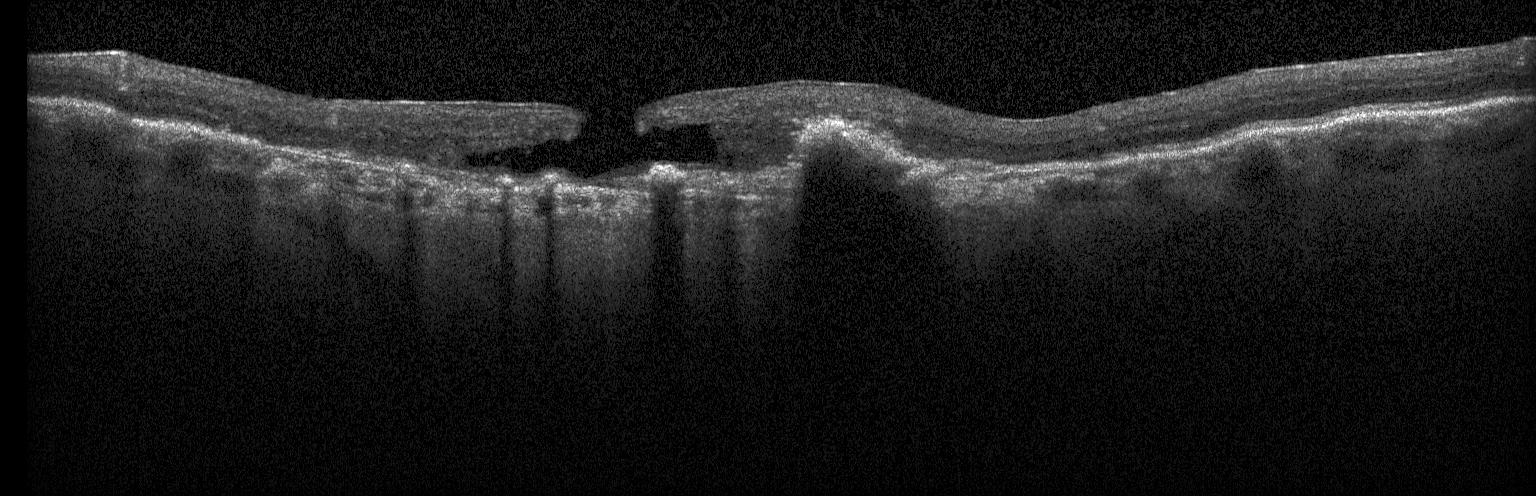
A choroidal neovascular membrane.